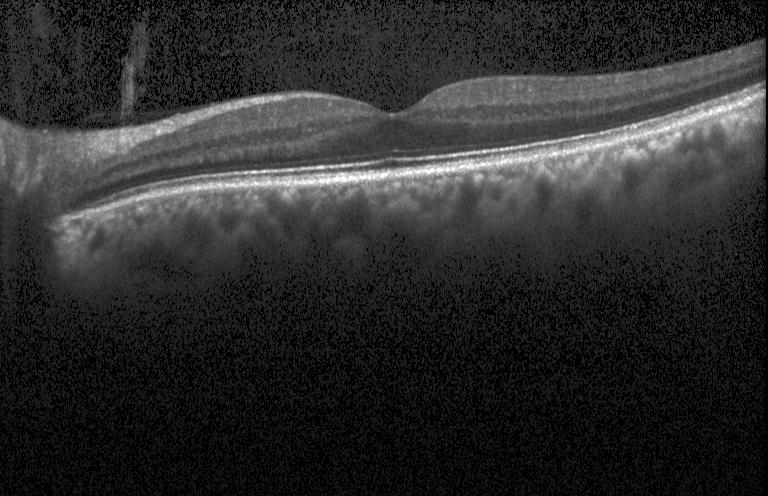 OCT B-scan — Finding: no evidence of choroidal neovascularization, diabetic macular edema, or drusen.